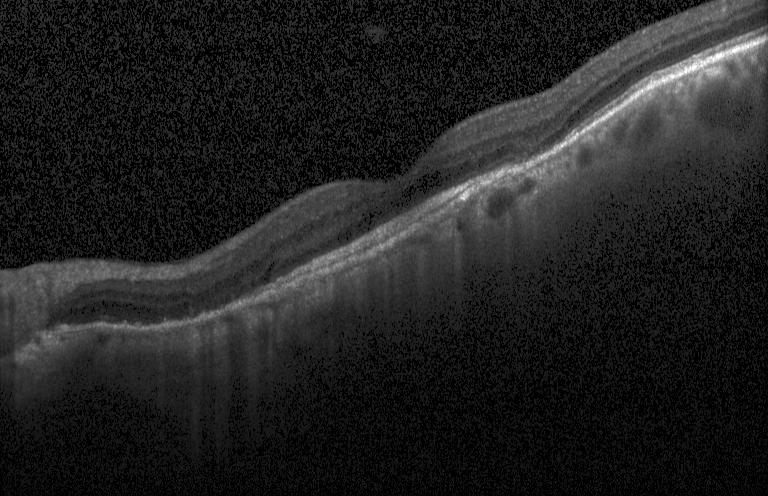
OCT B-scan
The scan shows a choroidal neovascular membrane.